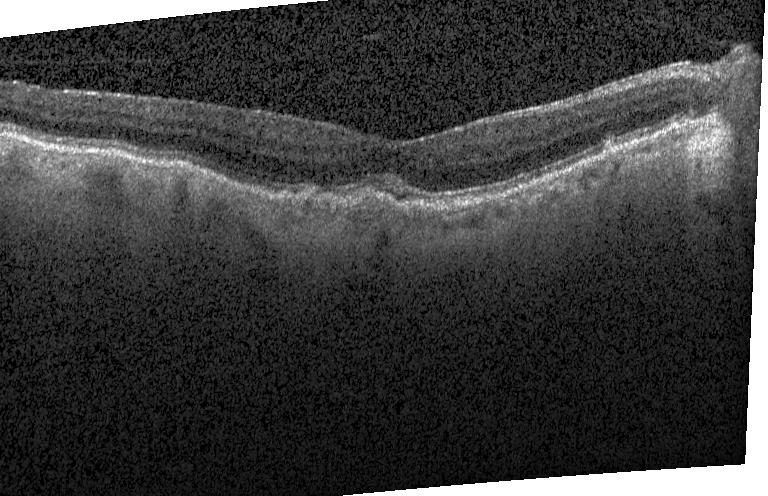
OCT scan showing choroidal neovascularization (CNV).